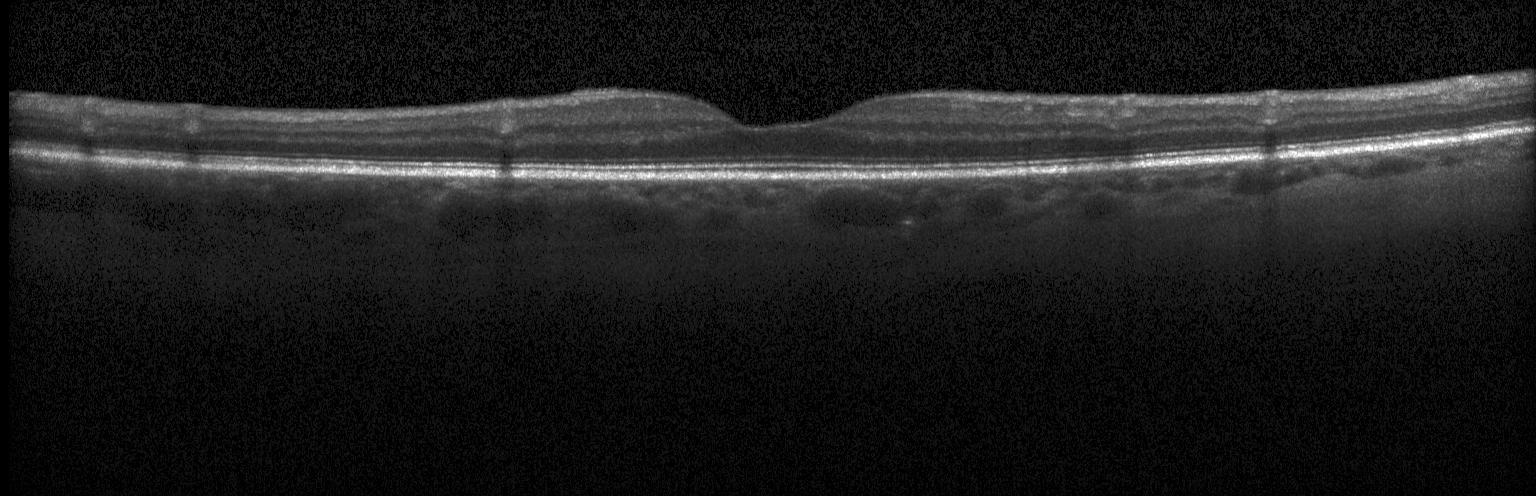
OCT finding: no evidence of choroidal neovascularization, diabetic macular edema, or drusen.